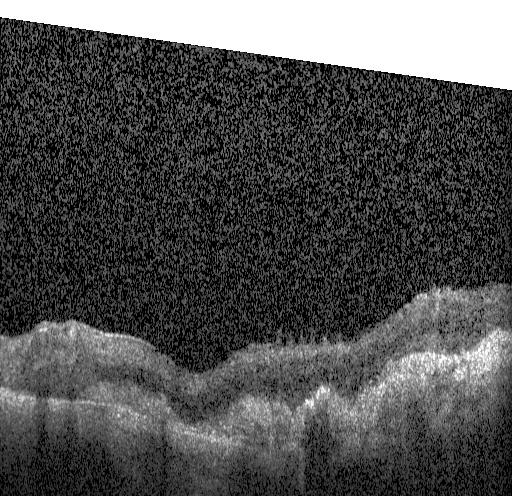

CNV.